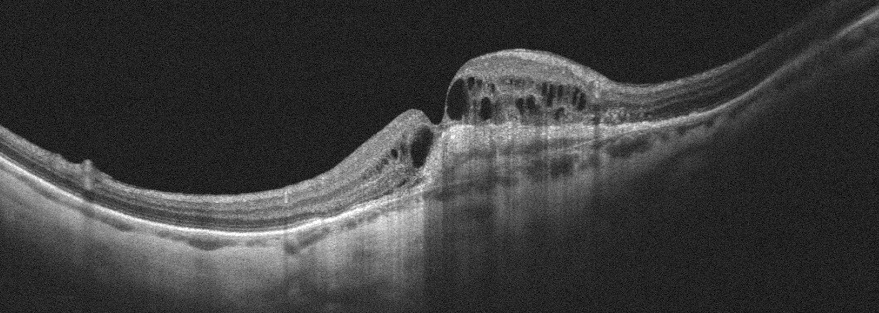

Macular scan, optical coherence tomography B-scan
Macular OCT: age-related macular degeneration (AMD).